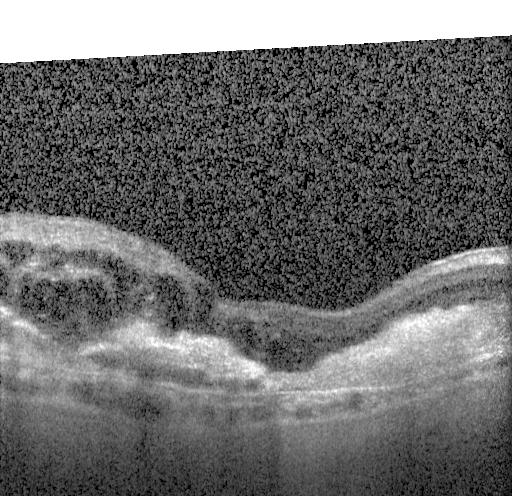

Retinal OCT B-scan, spectral-domain optical coherence tomography — Diagnosis: a choroidal neovascular membrane.